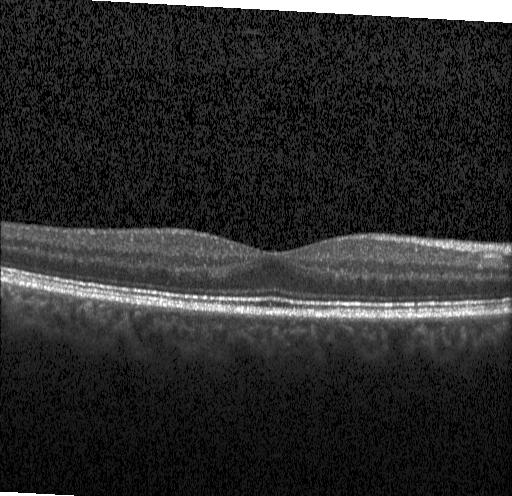 Impression: no CNV, no DME, and no drusen.